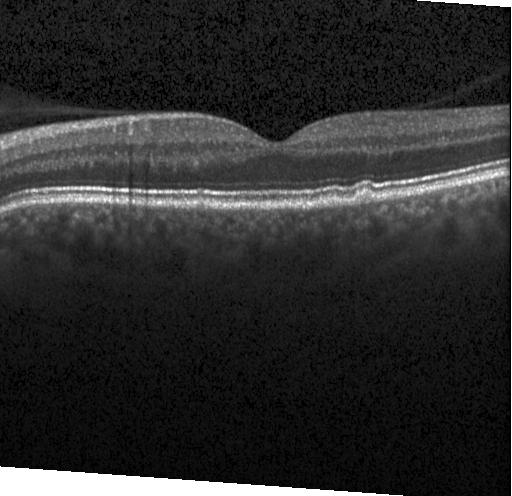 Through the macula. SD-OCT. OCT line scan
Impression: multiple drusen.